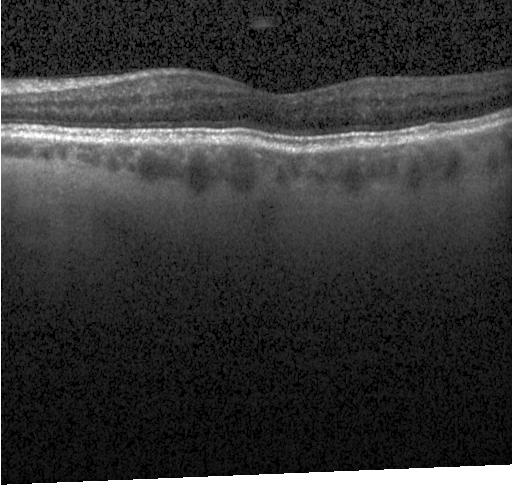

Impression: no choroidal neovascularization, diabetic macular edema, or drusen.